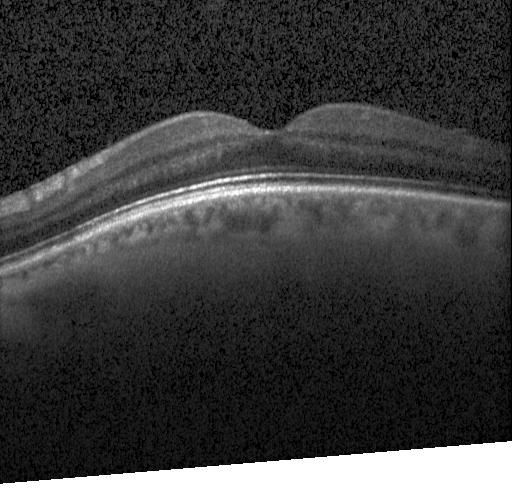
Retinal OCT cross-section — This B-scan demonstrates no CNV, no DME, and no drusen.